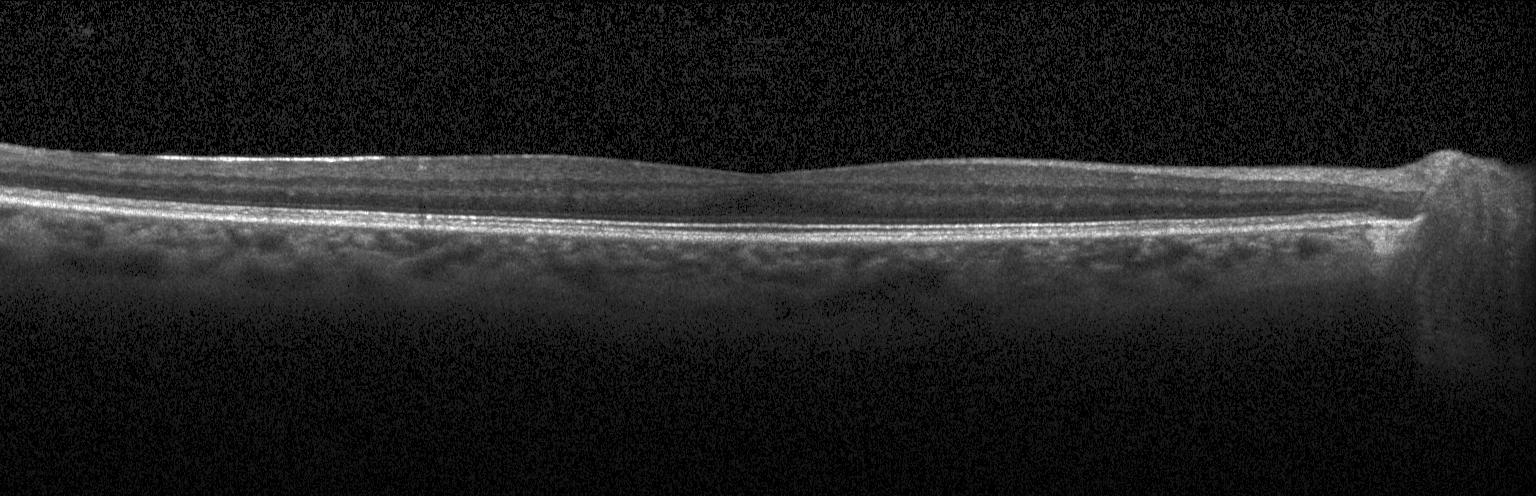

Macular OCT demonstrating no CNV, DME, or drusen.